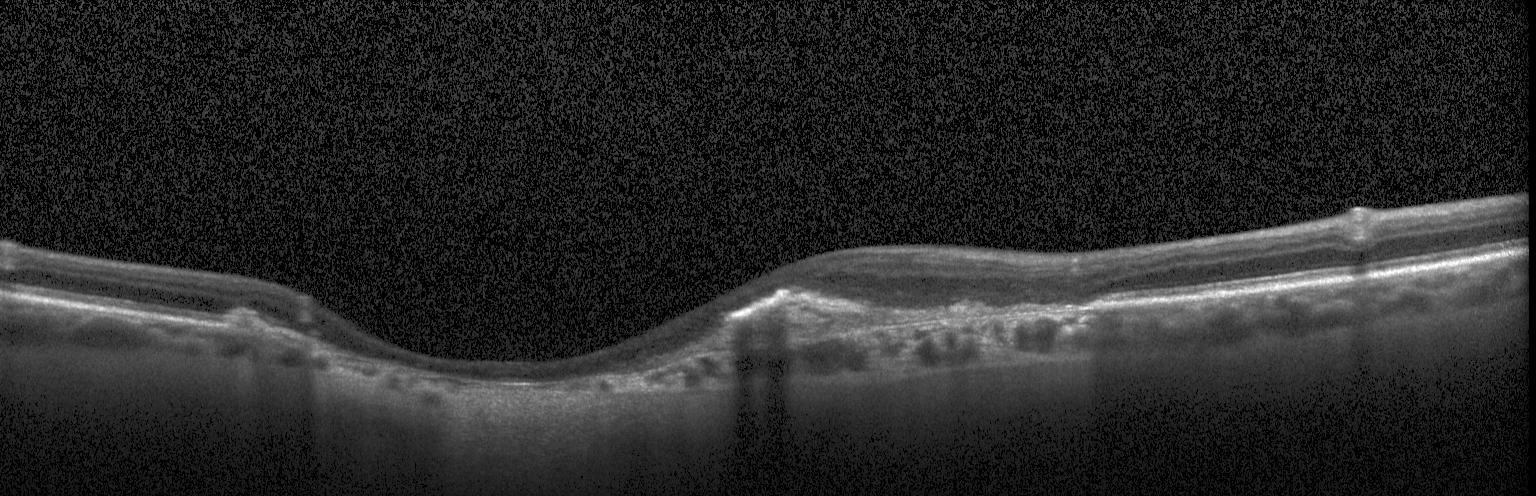 Macular OCT: a choroidal neovascular membrane.